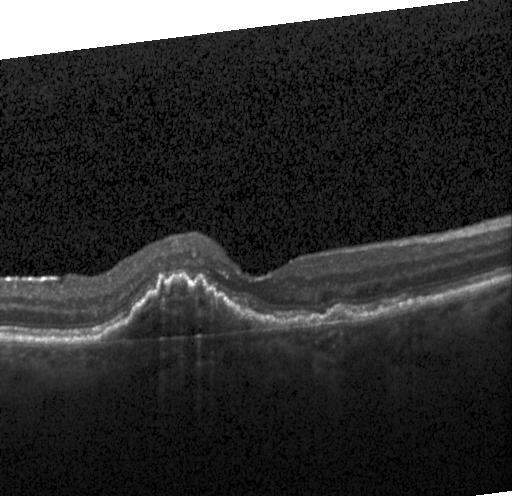
Retinal OCT B-scan; through the macula; spectral-domain optical coherence tomography; acquired on a Heidelberg Spectralis
Finding: a choroidal neovascular membrane.